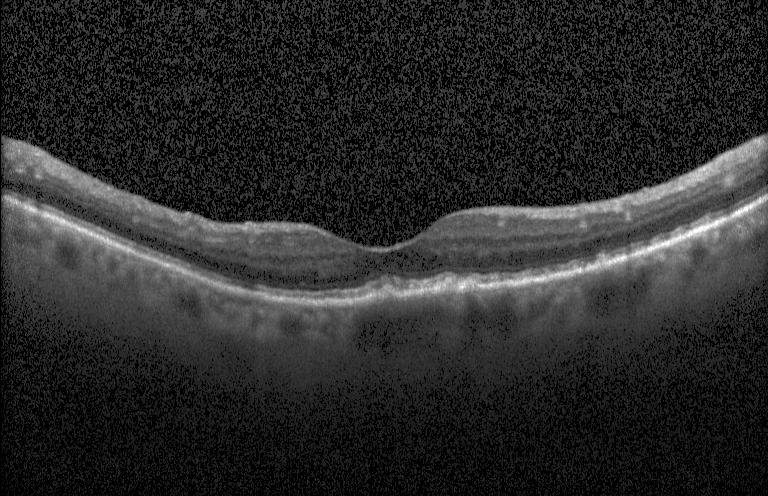 The scan shows sub-RPE drusenoid deposits.